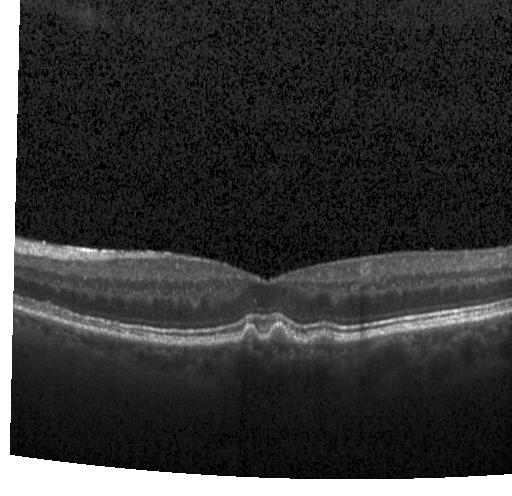 Optical coherence tomography B-scan.
Dx: multiple drusen.